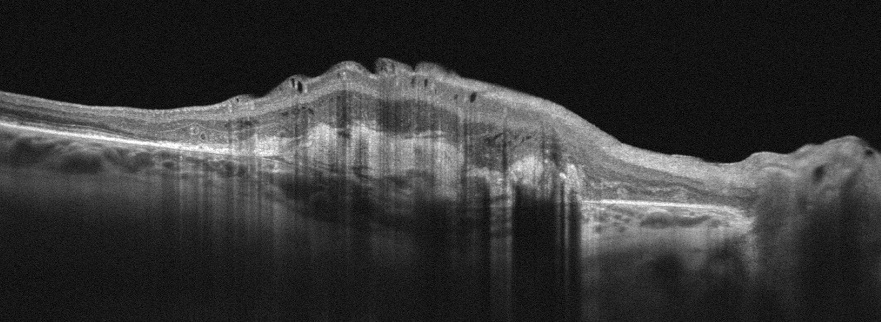
OCT B-scan. The scan shows AMD.